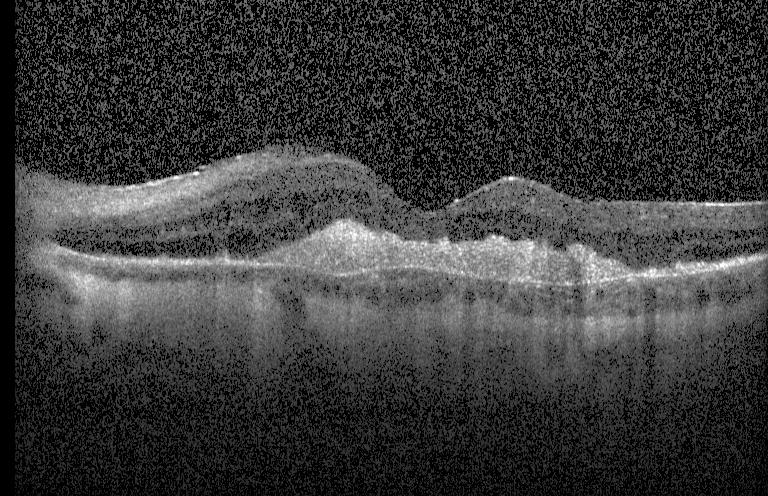

Finding: a choroidal neovascular membrane.